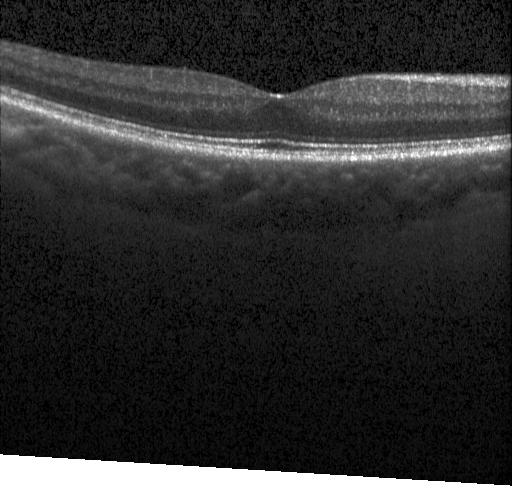 Centered on the fovea; optical coherence tomography B-scan.
No choroidal neovascularization, no diabetic macular edema, and no drusen.